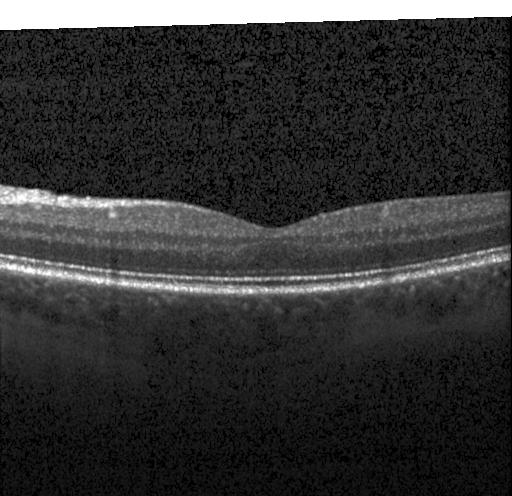

OCT B-scan showing no evidence of choroidal neovascularization, diabetic macular edema, or drusen.